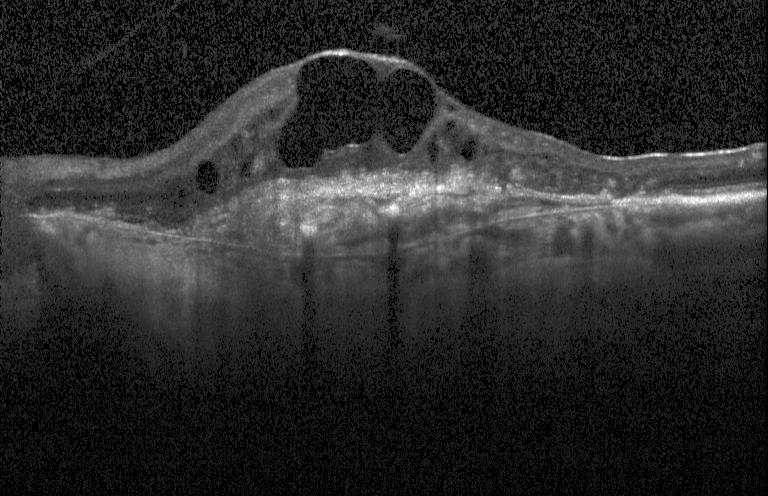
Macular OCT demonstrating a choroidal neovascular membrane.